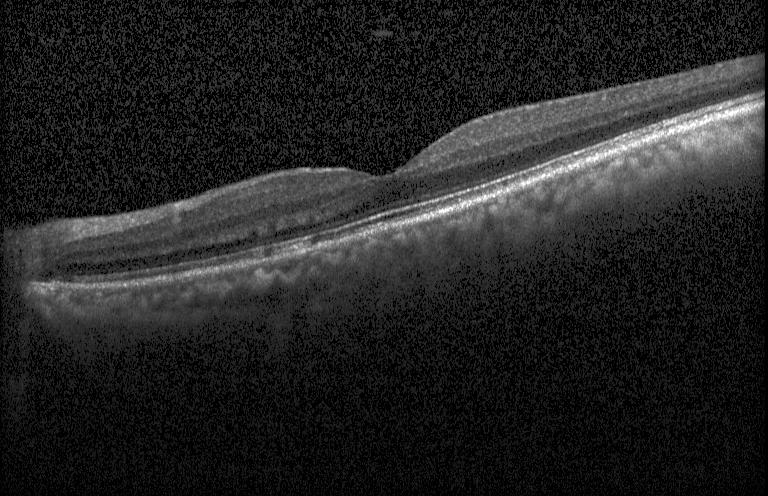
OCT finding: no choroidal neovascularization, diabetic macular edema, or drusen.